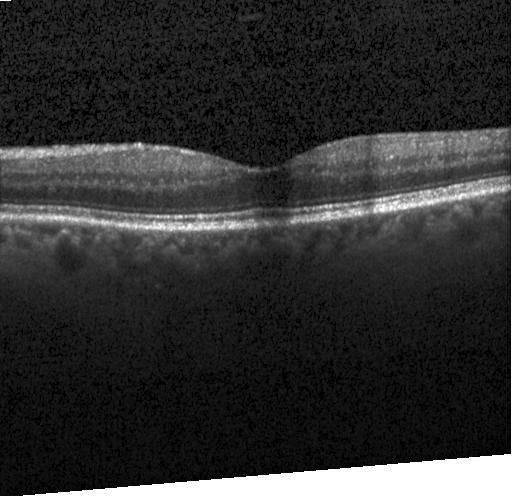 Optical coherence tomography B-scan. The scan shows no choroidal neovascularization, diabetic macular edema, or drusen.